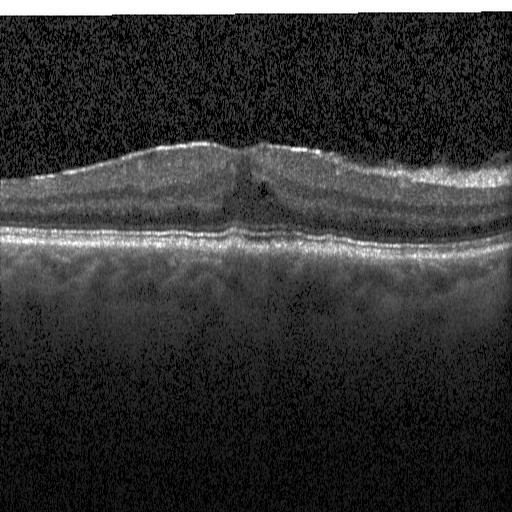
OCT scan showing diabetic macular edema (DME).